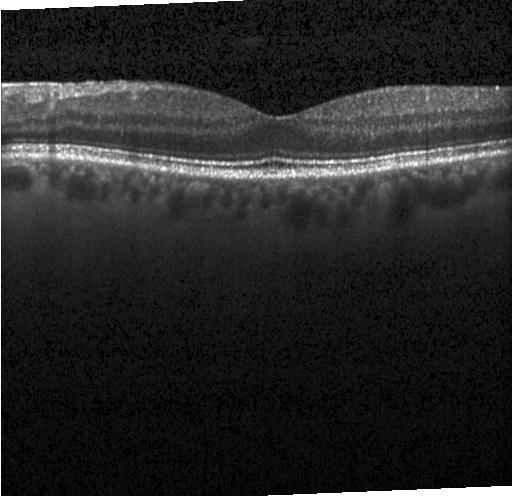

Fovea-centered; Heidelberg Spectralis; OCT line scan — Finding: no evidence of CNV, DME, or drusen.